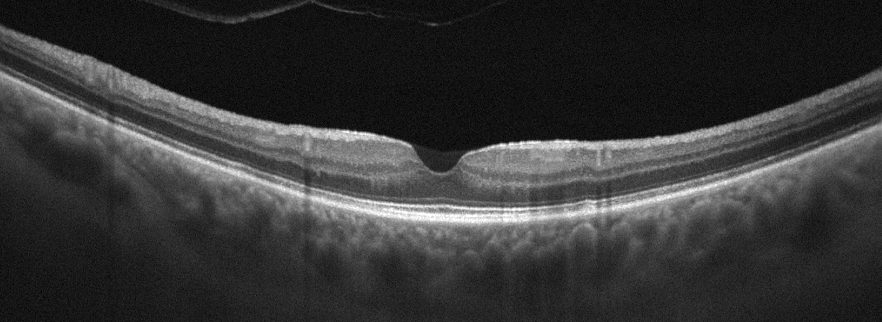
Instrument: Optovue Avanti RTVue XR; OCT B-scan; right eye; macular scan
Epiretinal membrane.